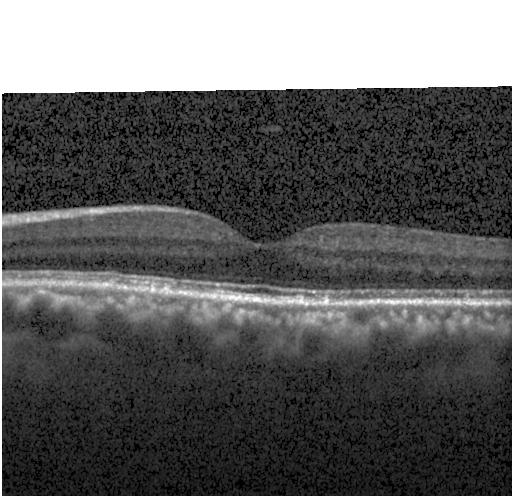
Finding: no choroidal neovascularization, diabetic macular edema, or drusen.